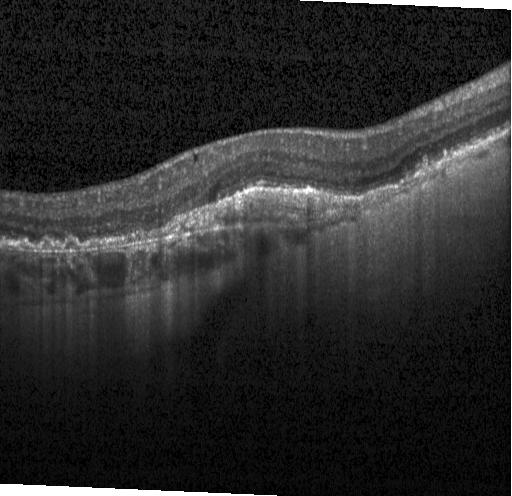 Retinal OCT B-scan — Assessment: choroidal neovascularization.